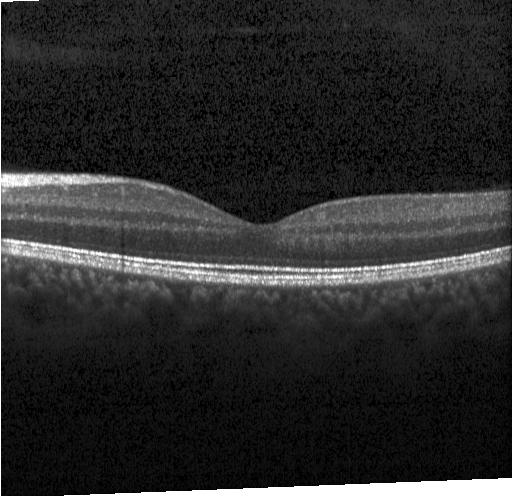
Finding: no evidence of CNV, DME, or drusen.